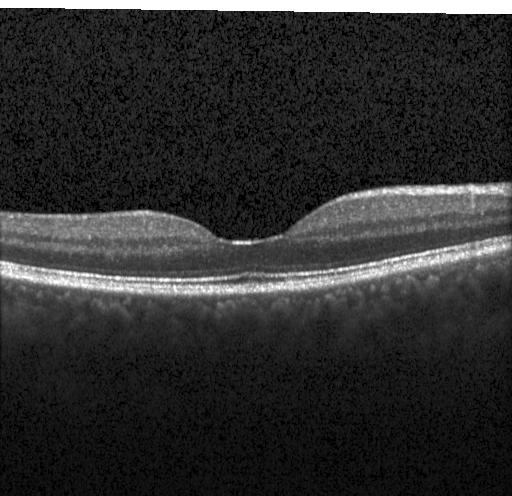
Spectral-domain optical coherence tomography. Optical coherence tomography scan. Heidelberg Spectralis OCT system — This B-scan demonstrates no choroidal neovascularization, no diabetic macular edema, and no drusen.